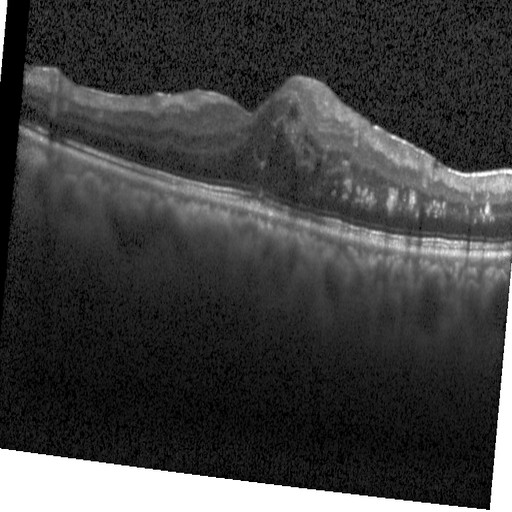
Macular scan · retinal OCT cross-section · spectral-domain OCT · Heidelberg Spectralis OCT system.
Finding: DME.